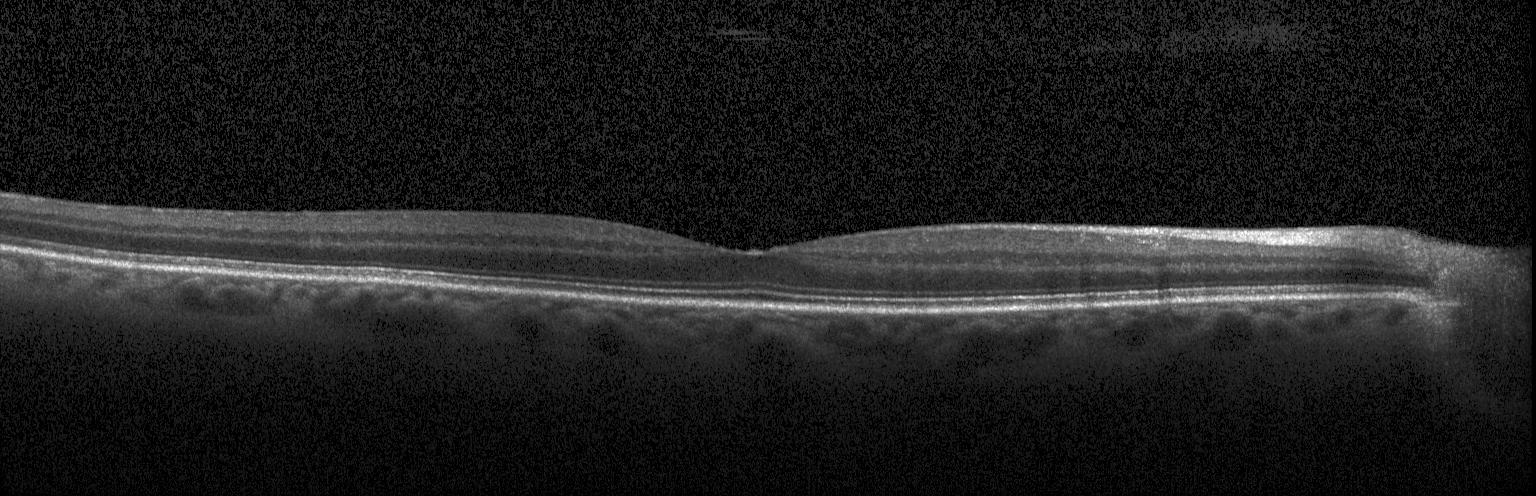

OCT line scan.
Diagnosis: neither CNV, DME, nor drusen.